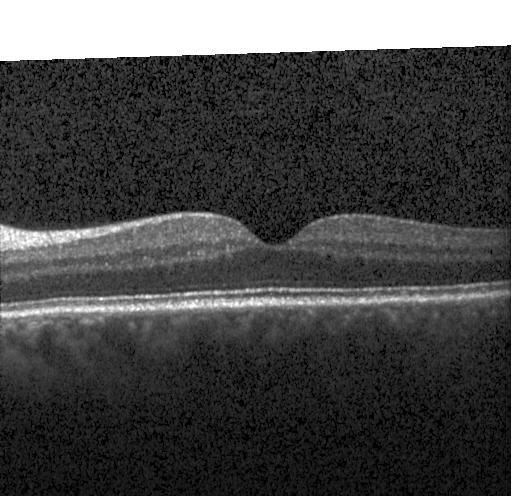

OCT B-scan showing no choroidal neovascularization, diabetic macular edema, or drusen.